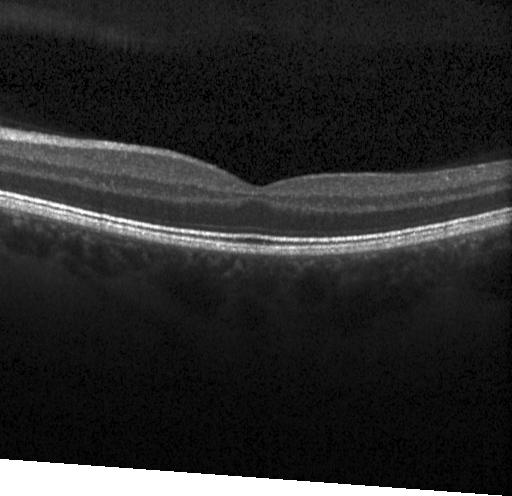

Retinal OCT cross-section showing no evidence of CNV, DME, or drusen.